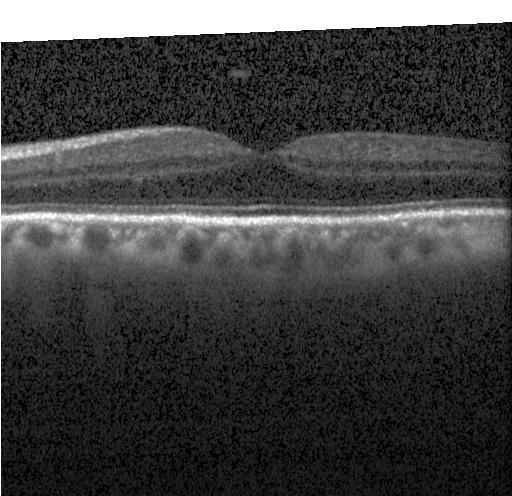
Spectral-domain OCT. Heidelberg Spectralis OCT system. Horizontal scan through the fovea. Optical coherence tomography scan — Impression: no CNV, no DME, and no drusen.